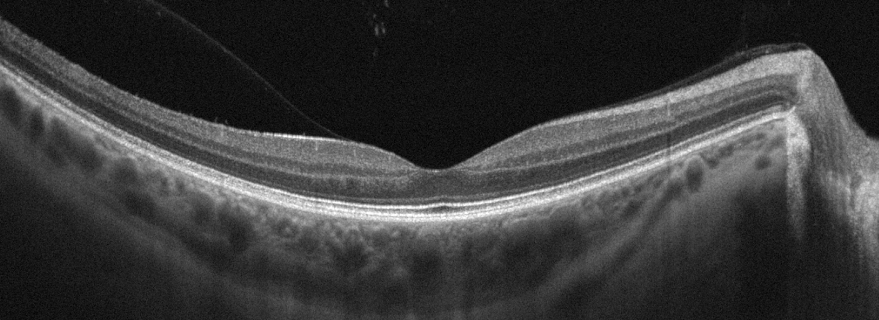 Retinal OCT cross-section. Impression: no evidence of AMD, DME, ERM, RAO, RVO, or VID.